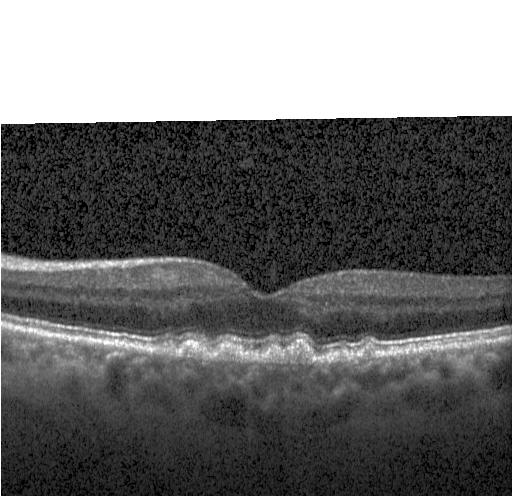

Heidelberg Spectralis. Optical coherence tomography B-scan. Spectral-domain OCT. Fovea-centered
This B-scan demonstrates sub-RPE drusenoid deposits.